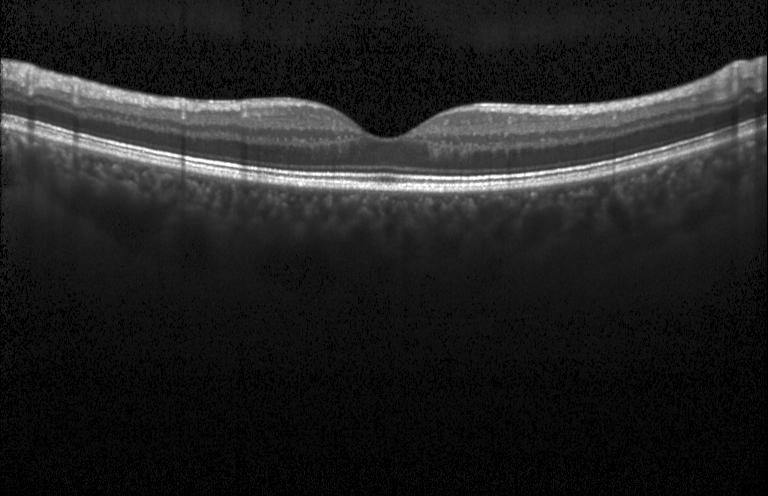 Through the macula · optical coherence tomography B-scan · spectral-domain OCT.
The scan shows no evidence of choroidal neovascularization, diabetic macular edema, or drusen.